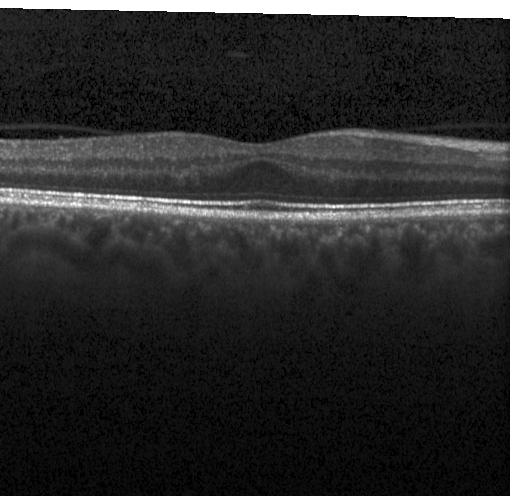 Optical coherence tomography scan, centered on the fovea, spectral-domain OCT, Heidelberg Spectralis OCT system. This B-scan demonstrates no choroidal neovascularization, no diabetic macular edema, and no drusen.